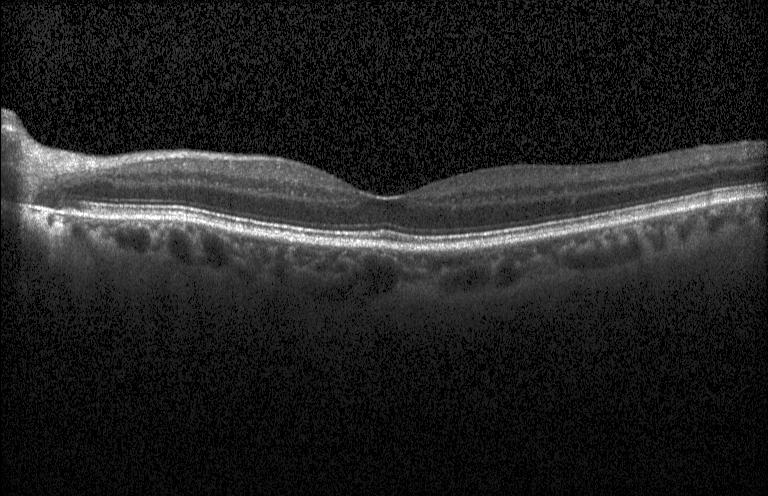

SD-OCT, fovea-centered, optical coherence tomography B-scan. Assessment: neither choroidal neovascularization, diabetic macular edema, nor drusen.